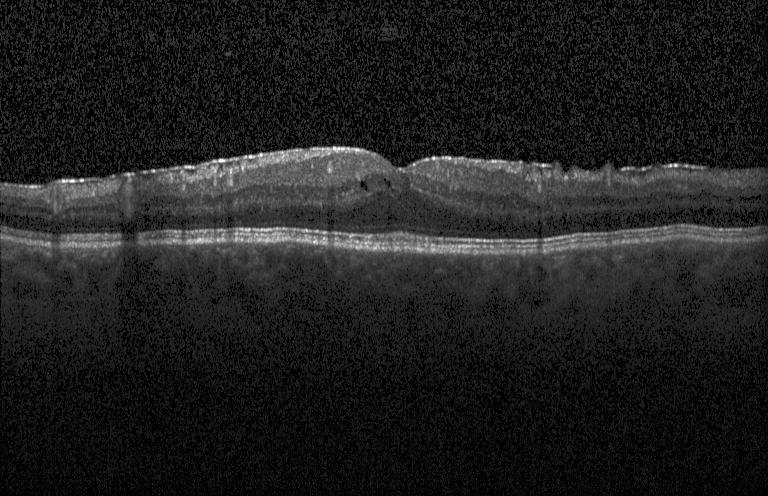
OCT finding: diabetic macular edema (DME).